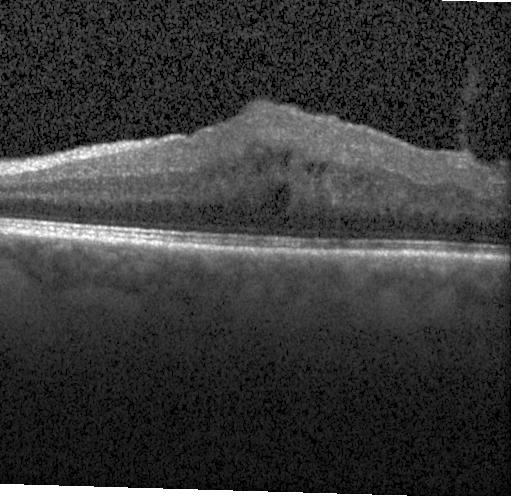

OCT B-scan.
Impression: diabetic macular edema (DME).